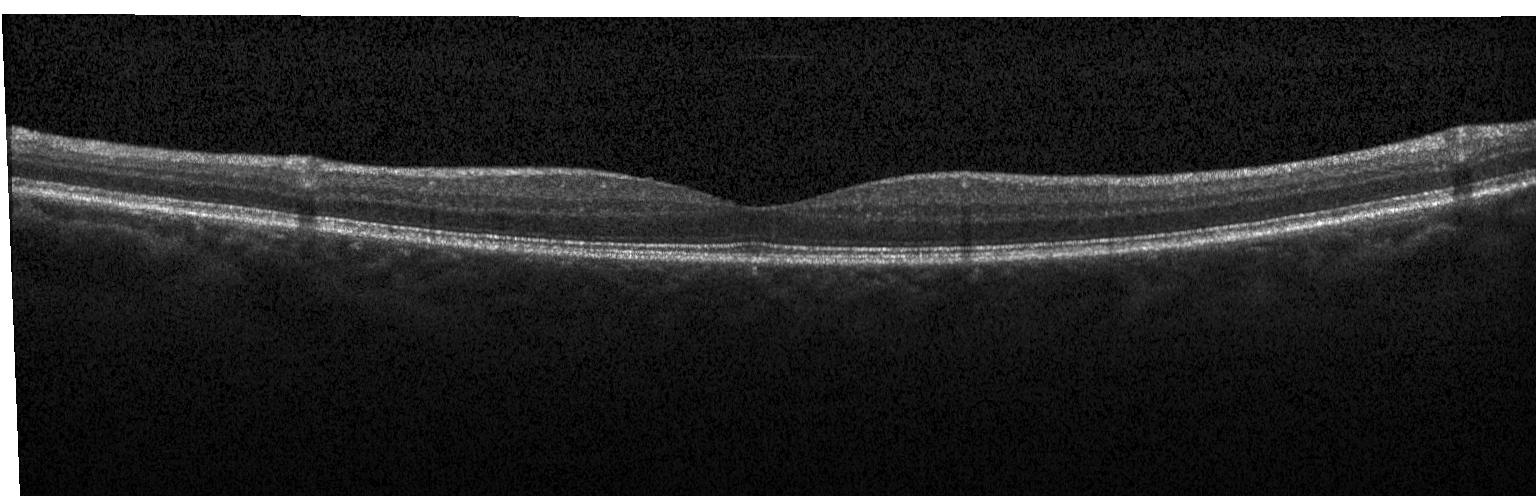

Spectral-domain OCT, OCT line scan.
Macular OCT: no evidence of choroidal neovascularization, diabetic macular edema, or drusen.